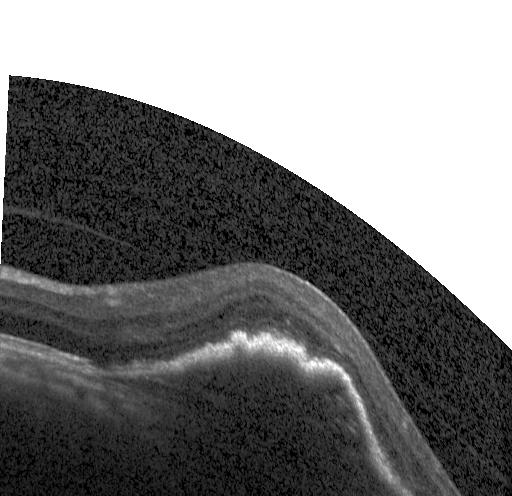 The scan shows CNV.